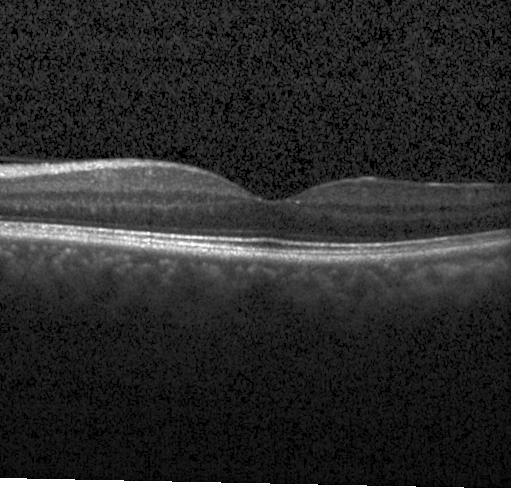 OCT B-scan.
This B-scan demonstrates no choroidal neovascularization, no diabetic macular edema, and no drusen.